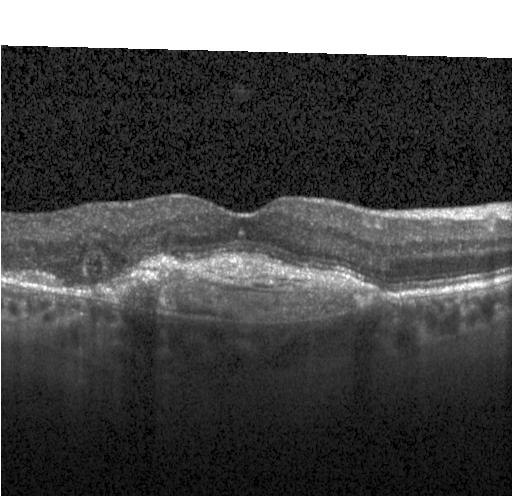
Optical coherence tomography scan; spectral-domain OCT; centered on the fovea; instrument: Heidelberg Spectralis — Impression: a choroidal neovascular membrane.